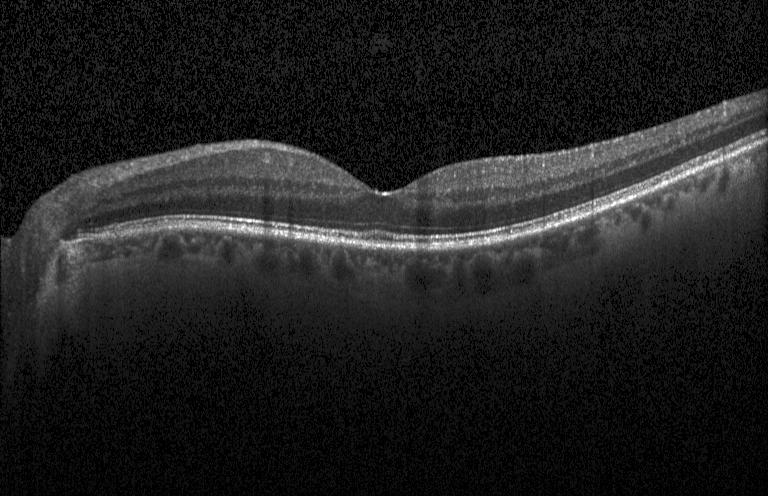
Macular scan, SD-OCT, Heidelberg Spectralis OCT system, retinal OCT B-scan.
Diagnosis: no evidence of choroidal neovascularization, diabetic macular edema, or drusen.